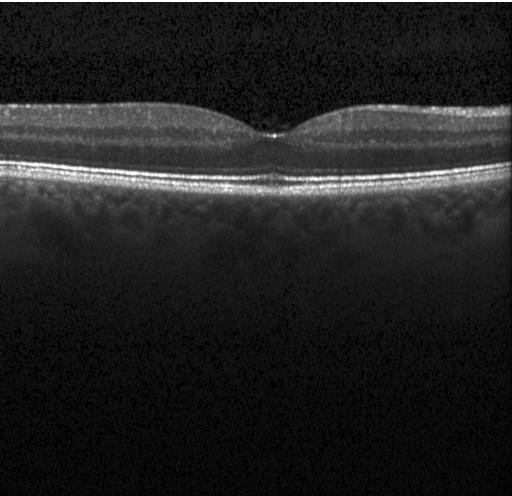 Retinal OCT B-scan. Instrument: Heidelberg Spectralis. SD-OCT.
This B-scan demonstrates no choroidal neovascularization, no diabetic macular edema, and no drusen.